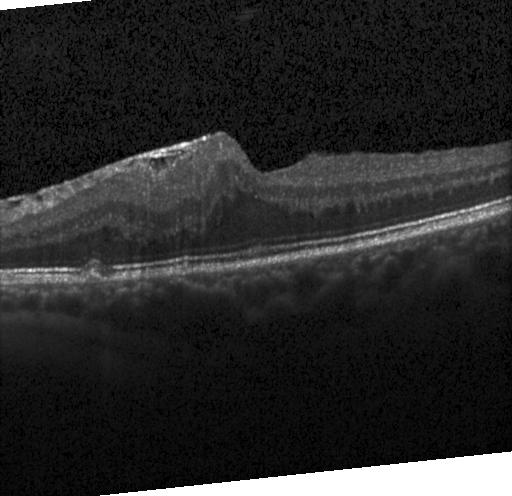 SD-OCT. Macular scan. Retinal OCT cross-section. Impression: drusen.